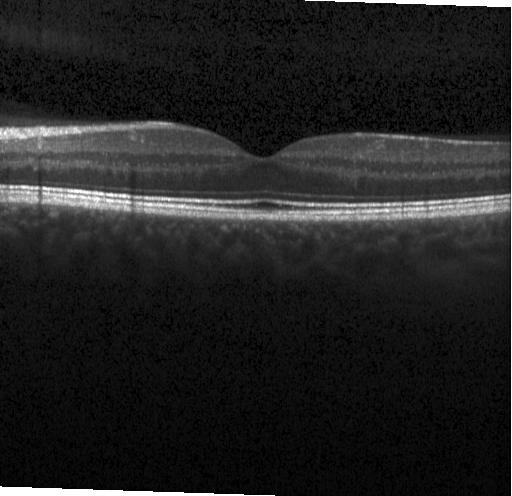 Optical coherence tomography scan.
Finding: no evidence of choroidal neovascularization, diabetic macular edema, or drusen.